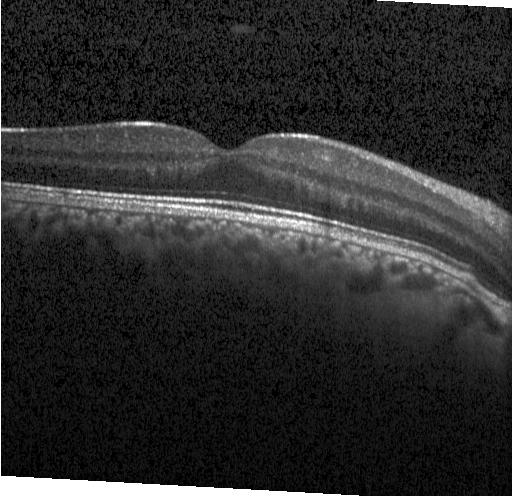 This B-scan demonstrates neither choroidal neovascularization, diabetic macular edema, nor drusen.